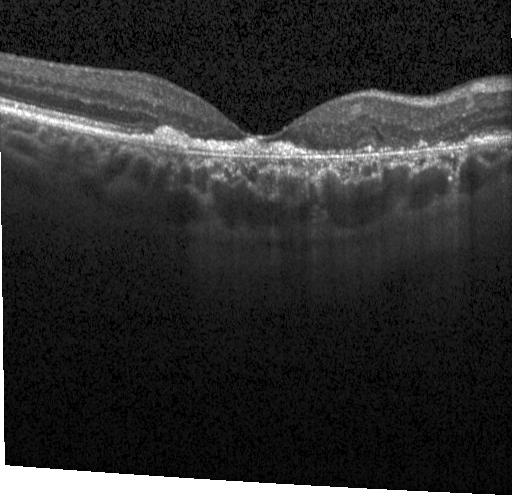
Spectral-domain optical coherence tomography; OCT line scan; fovea-centered; acquired on a Heidelberg Spectralis
Assessment: a choroidal neovascular membrane.